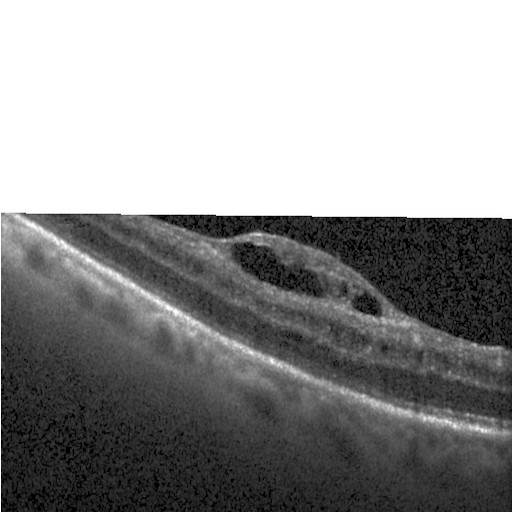
Instrument: Heidelberg Spectralis; optical coherence tomography scan.
Impression: diabetic macular edema.